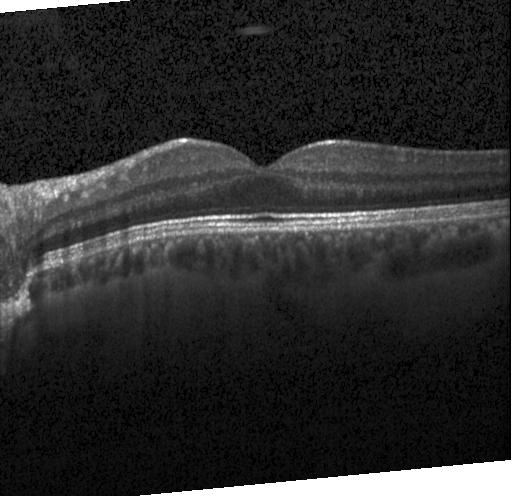

Retinal OCT cross-section. Diagnosis: neither choroidal neovascularization, diabetic macular edema, nor drusen.